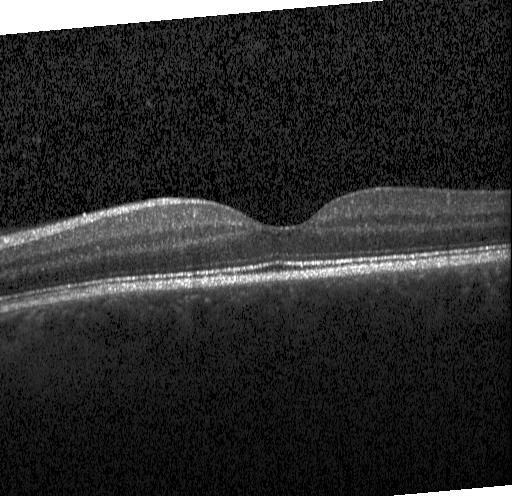

OCT line scan
Diagnosis: no evidence of choroidal neovascularization, diabetic macular edema, or drusen.